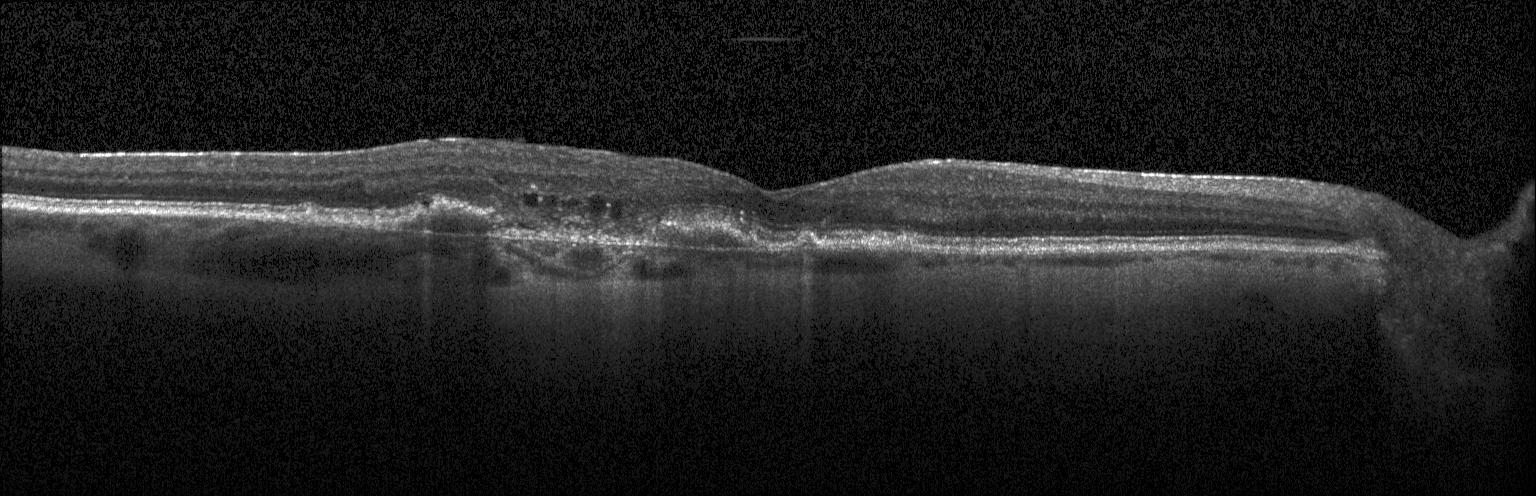 OCT scan showing choroidal neovascularization (CNV).